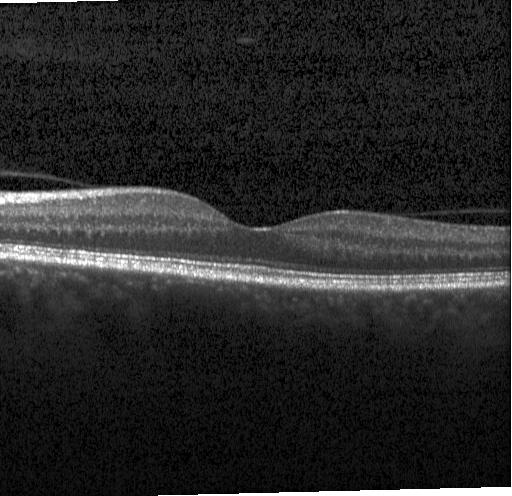 Retinal OCT B-scan
Macular OCT: no evidence of CNV, DME, or drusen.